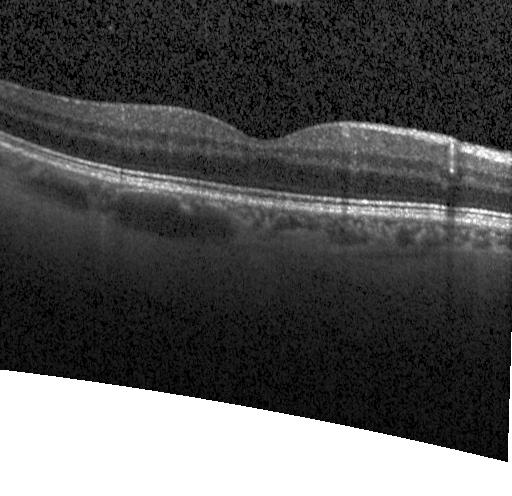

Heidelberg Spectralis OCT system, OCT line scan, macular scan.
OCT finding: no evidence of choroidal neovascularization, diabetic macular edema, or drusen.